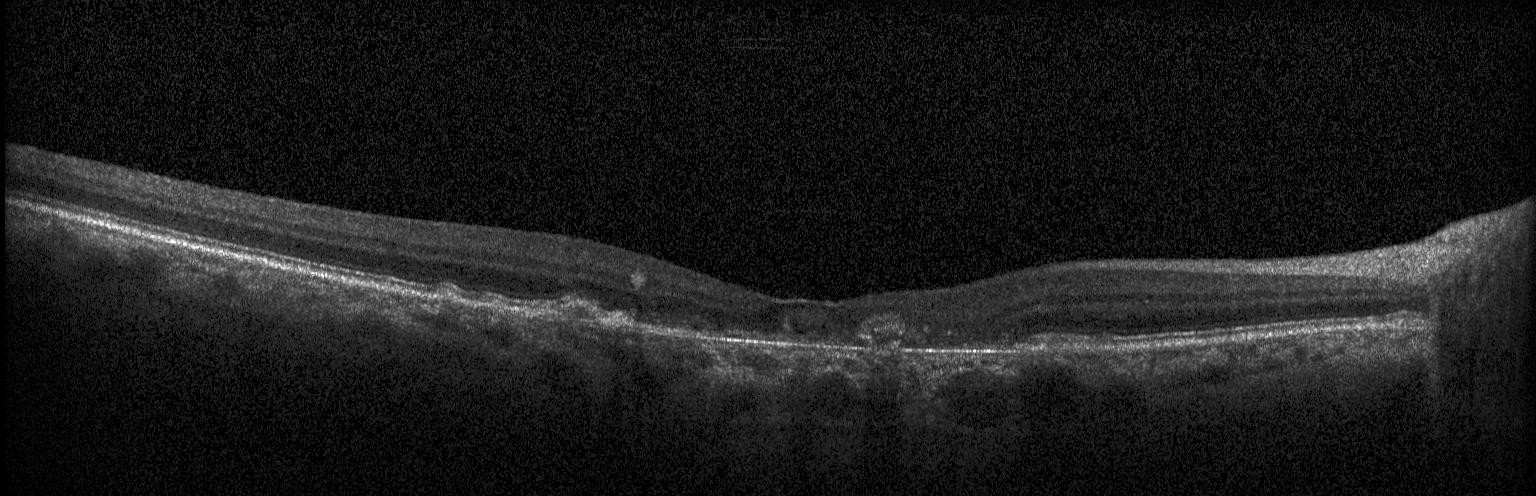

Macular OCT demonstrating choroidal neovascularization.